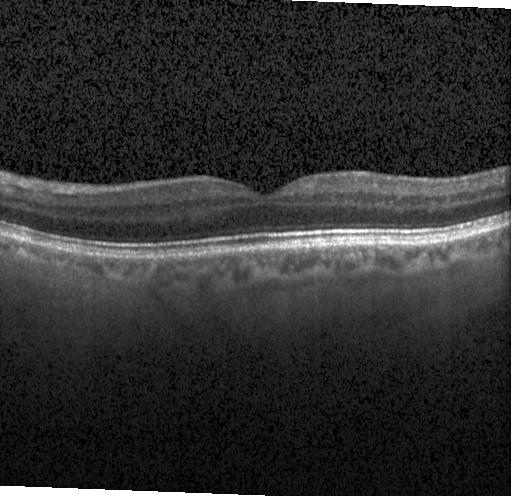

Heidelberg Spectralis. Spectral-domain optical coherence tomography. Retinal OCT B-scan.
Impression: no choroidal neovascularization, no diabetic macular edema, and no drusen.